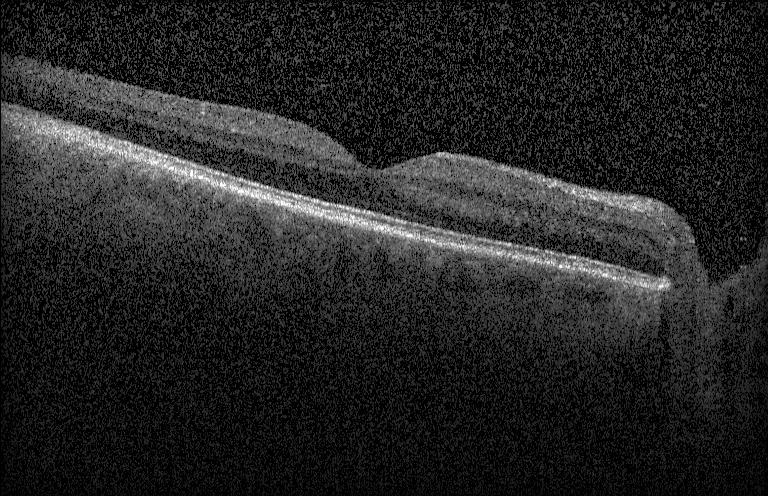
Retinal OCT B-scan. Instrument: Heidelberg Spectralis — Finding: no choroidal neovascularization, no diabetic macular edema, and no drusen.